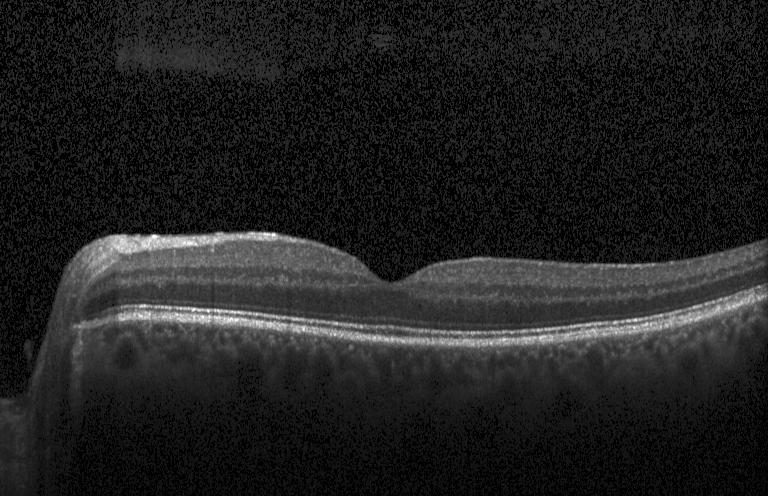

OCT line scan; Heidelberg Spectralis OCT system; SD-OCT; fovea-centered
Diagnosis: no choroidal neovascularization, no diabetic macular edema, and no drusen.